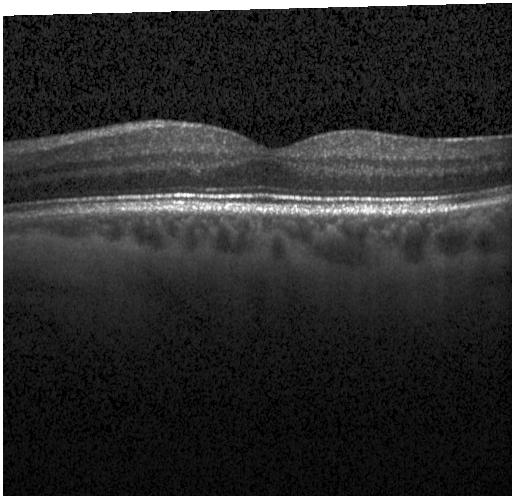
Through the macula · retinal OCT cross-section.
Finding: no choroidal neovascularization, no diabetic macular edema, and no drusen.